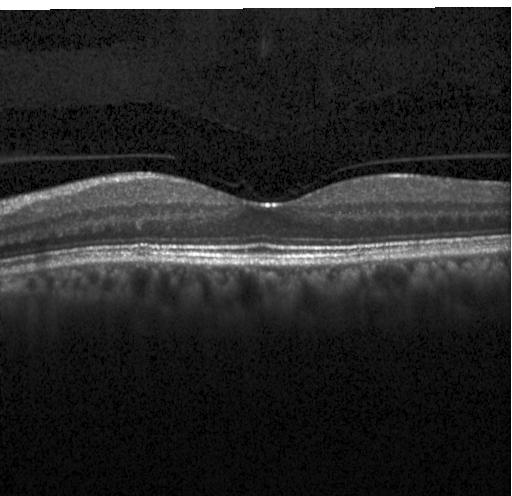 Impression: no choroidal neovascularization, no diabetic macular edema, and no drusen.